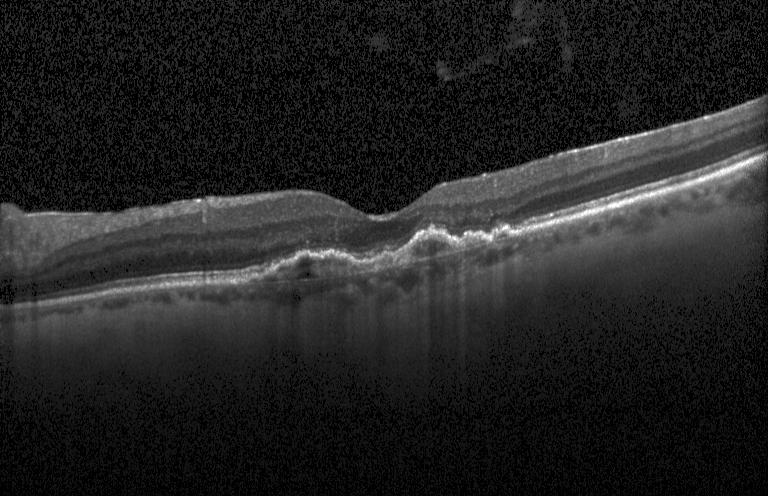

OCT finding: a choroidal neovascular membrane.